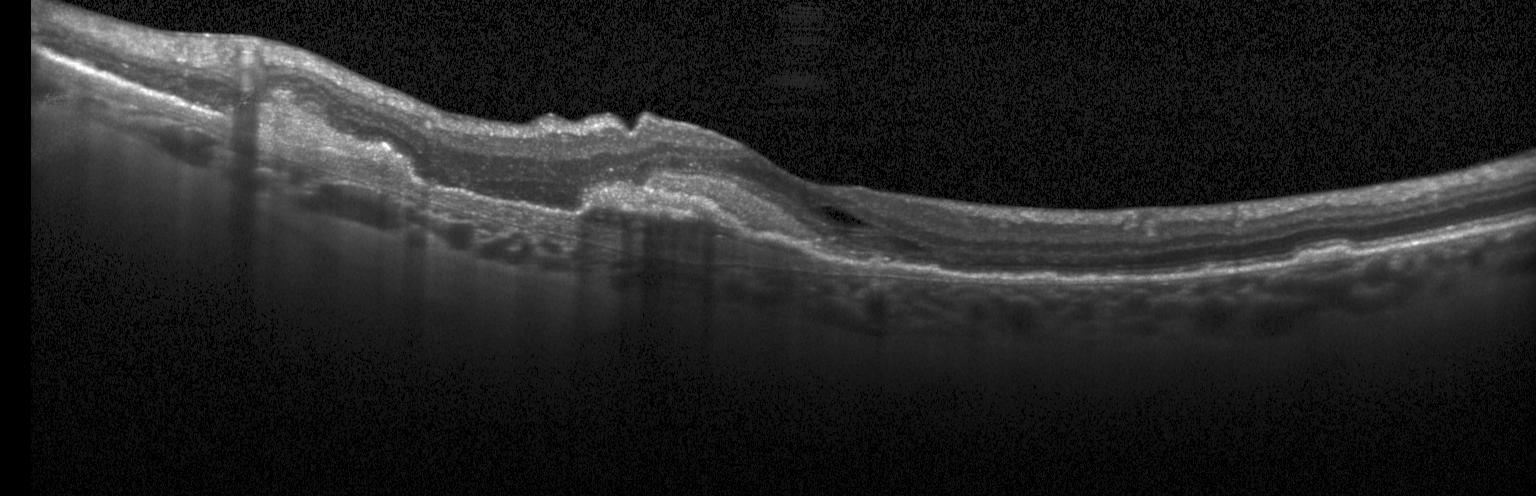 OCT B-scan. OCT finding: CNV.